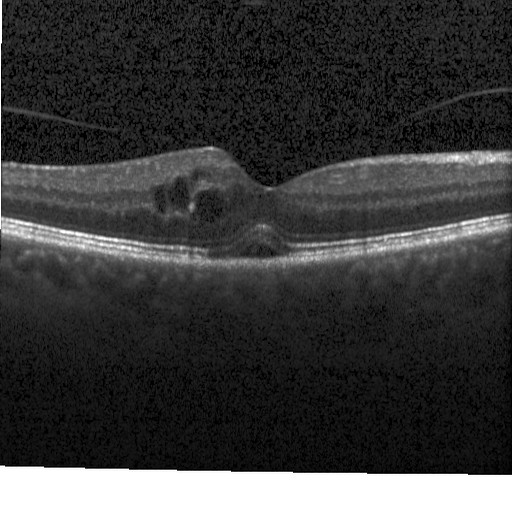
The scan shows diabetic macular edema.